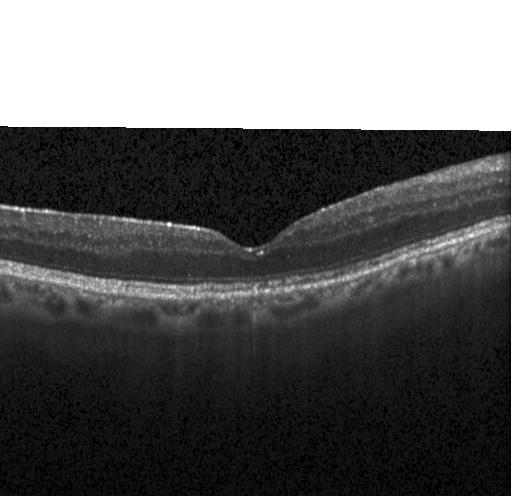
Acquired on a Heidelberg Spectralis. Retinal OCT B-scan
Assessment: neither CNV, DME, nor drusen.